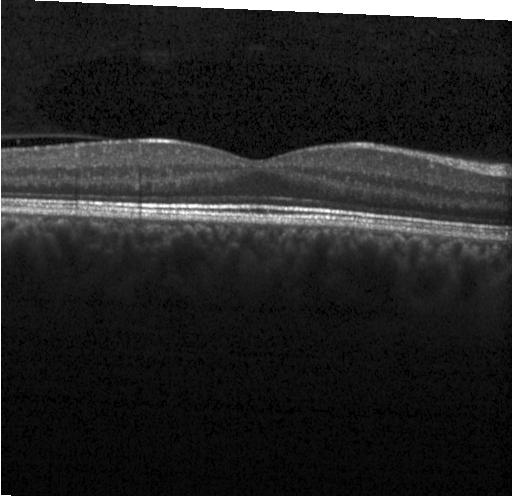 Acquired on a Heidelberg Spectralis, fovea-centered, spectral-domain OCT, optical coherence tomography B-scan. Assessment: neither choroidal neovascularization, diabetic macular edema, nor drusen.